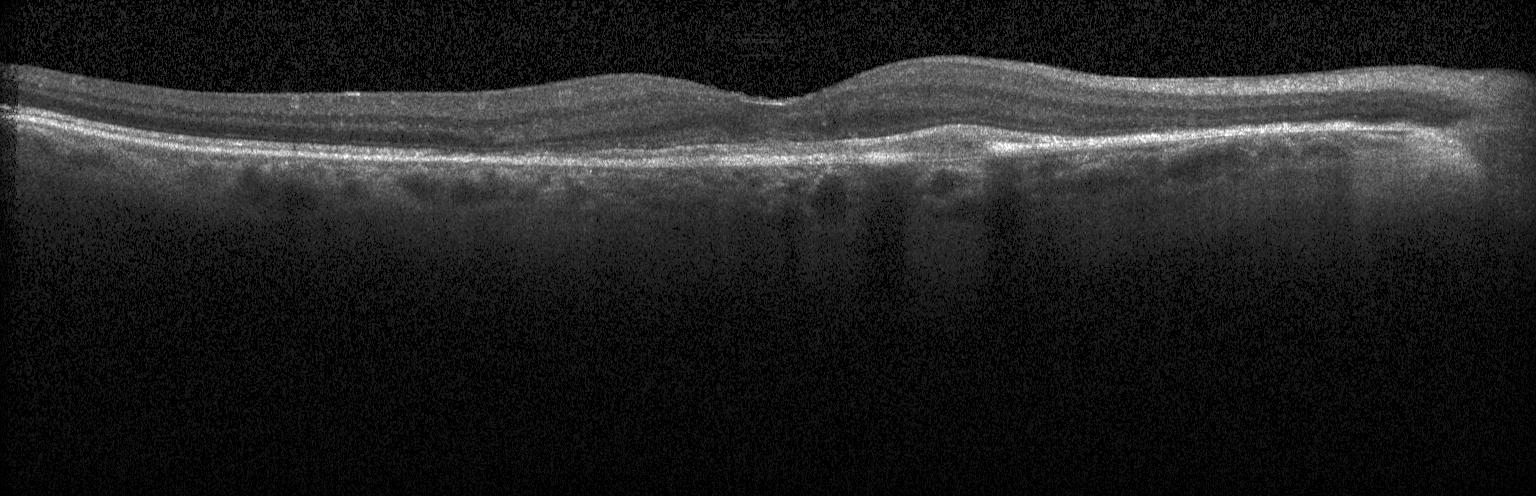
Retinal OCT cross-section showing choroidal neovascularization.